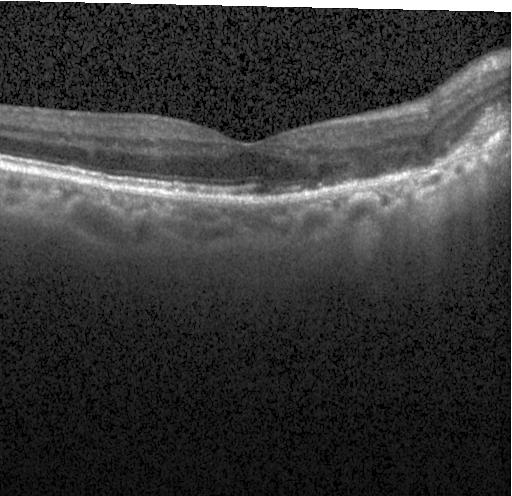

Impression: a choroidal neovascular membrane.